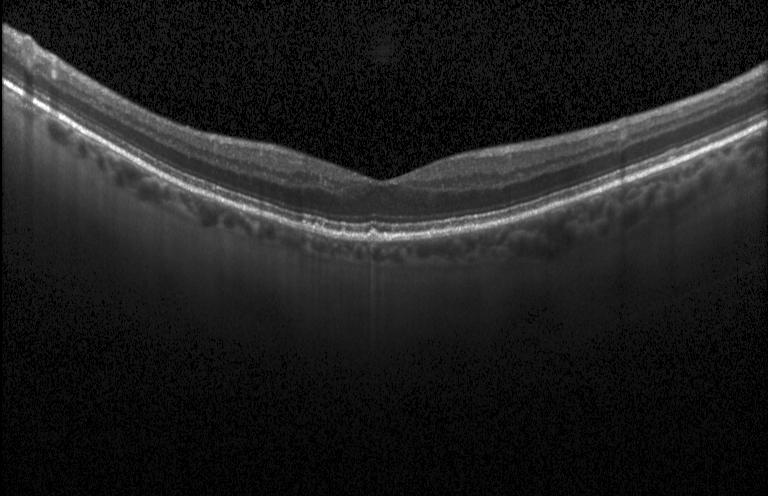
Spectral-domain optical coherence tomography. Retinal OCT B-scan. Through the macula. Heidelberg Spectralis — Diagnosis: multiple drusen.